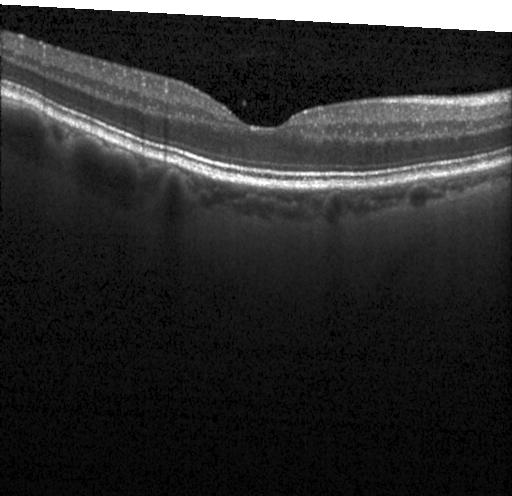 SD-OCT. OCT line scan. Horizontal scan through the fovea. Acquired on a Heidelberg Spectralis.
Impression: no choroidal neovascularization, no diabetic macular edema, and no drusen.